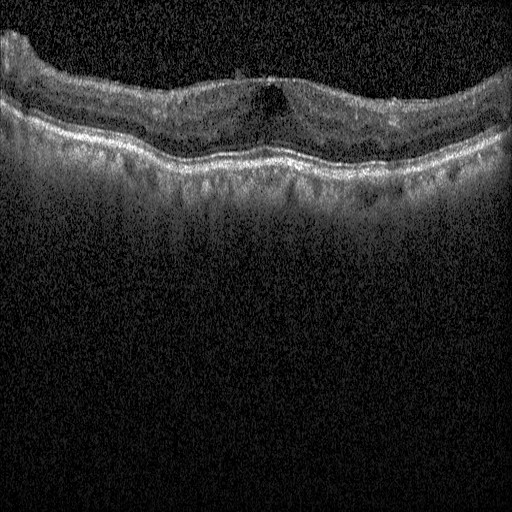
Impression: diabetic macular edema.